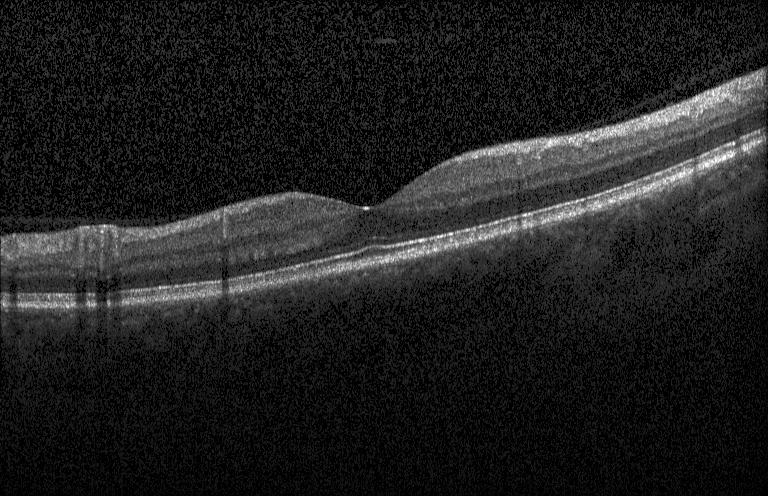
Assessment: neither choroidal neovascularization, diabetic macular edema, nor drusen.